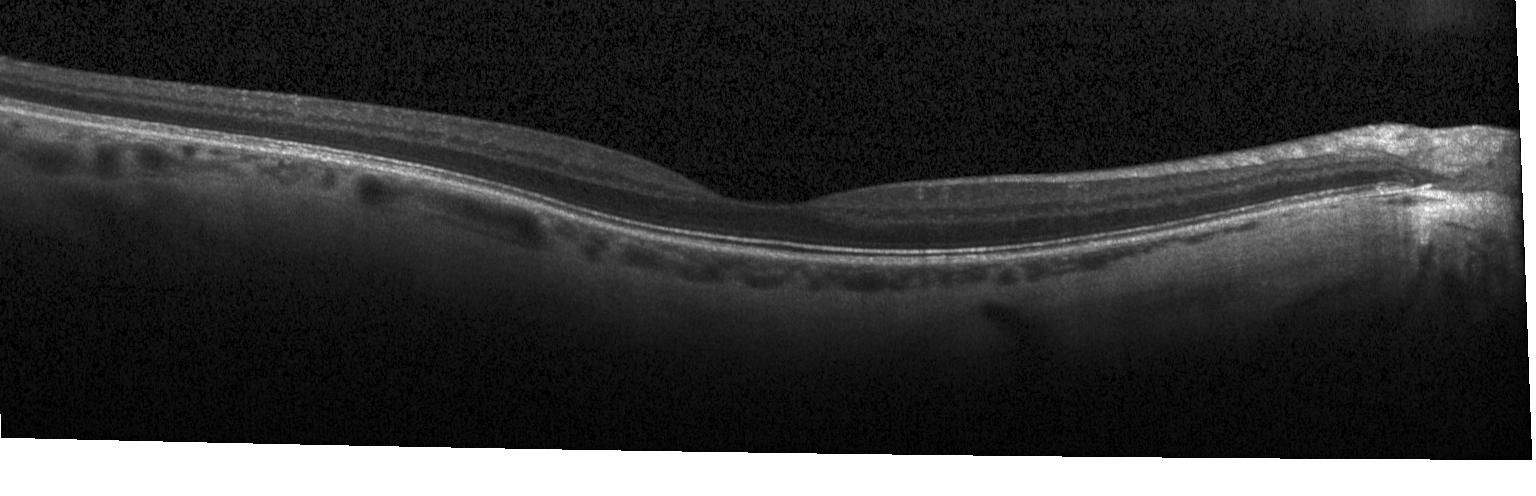 SD-OCT · retinal OCT cross-section.
This B-scan demonstrates no CNV, DME, or drusen.